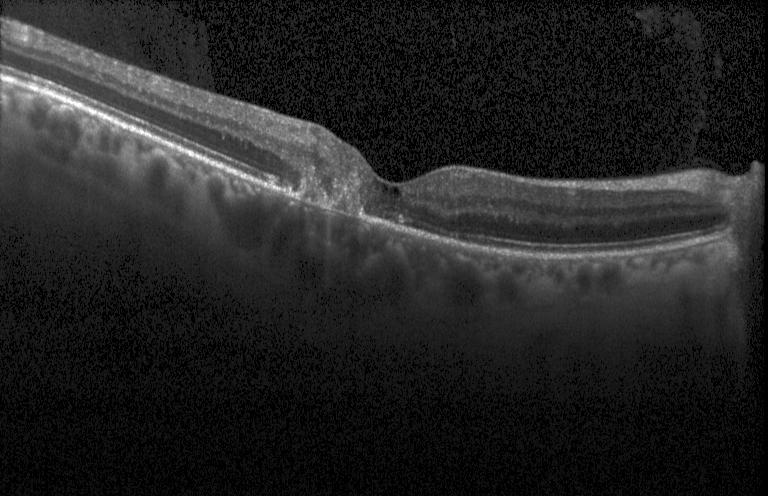
Finding: a choroidal neovascular membrane.